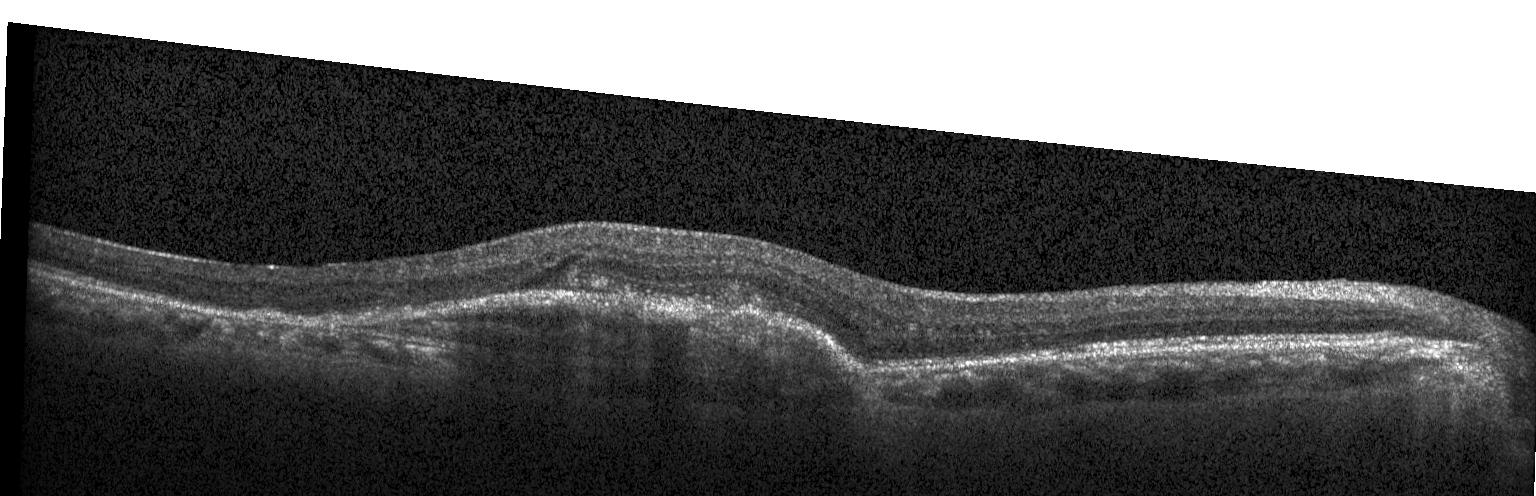 Finding: a choroidal neovascular membrane.